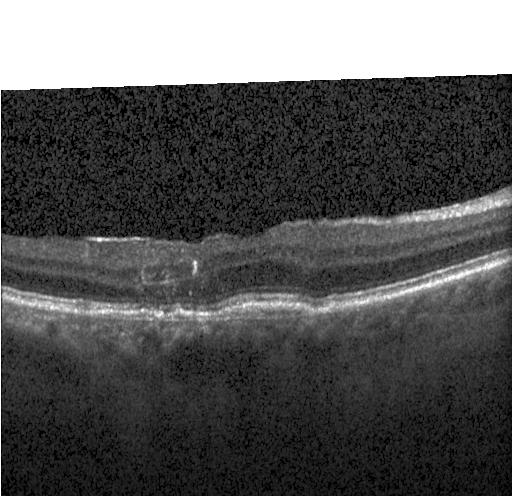 OCT line scan · SD-OCT · horizontal scan through the fovea — This B-scan demonstrates a choroidal neovascular membrane.